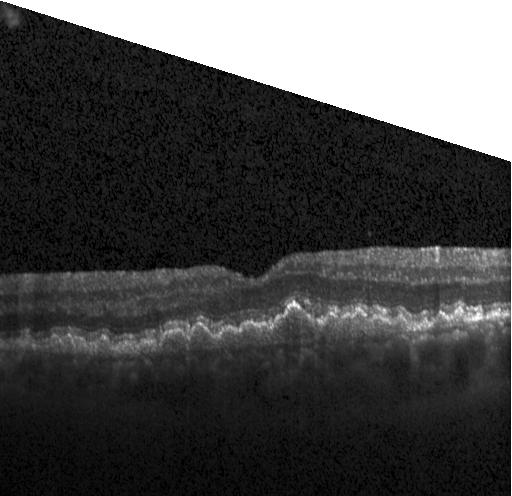 OCT line scan.
Macular OCT: choroidal neovascularization (CNV).